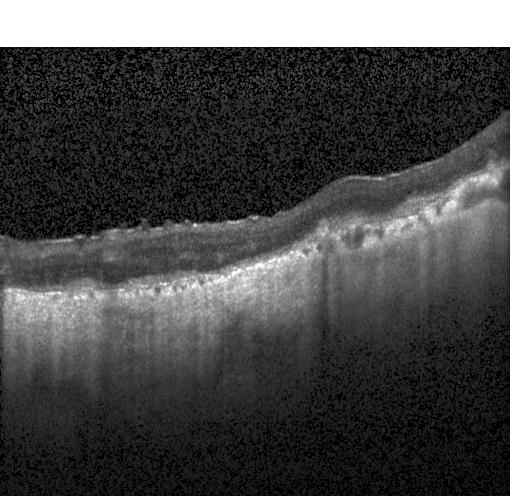 SD-OCT. Heidelberg Spectralis OCT system. Optical coherence tomography B-scan. Macular scan
This B-scan demonstrates CNV.